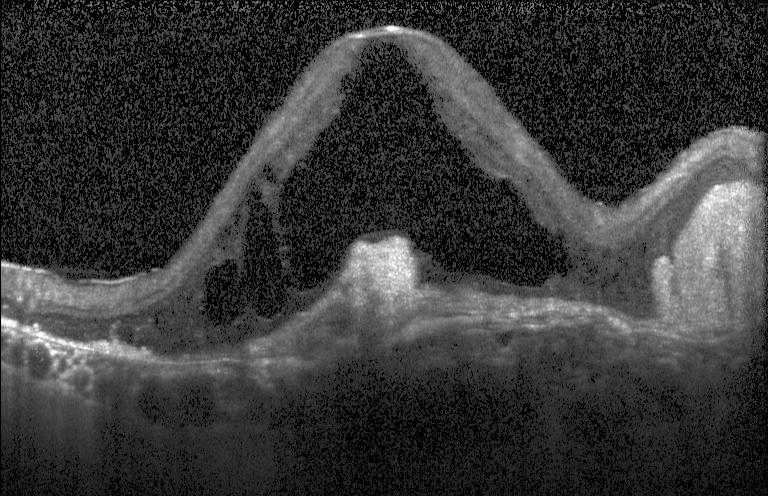 Retinal OCT cross-section. Diagnosis: choroidal neovascularization.